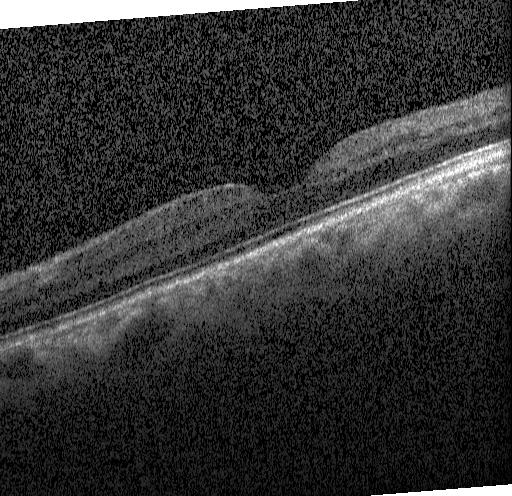
Assessment: no evidence of choroidal neovascularization, diabetic macular edema, or drusen.